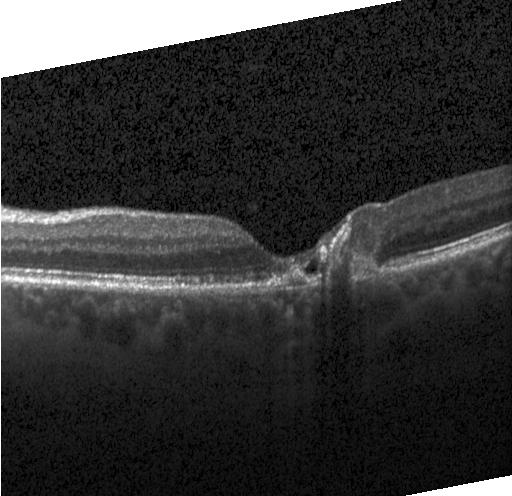

SD-OCT; instrument: Heidelberg Spectralis; horizontal scan through the fovea; OCT B-scan
Impression: a choroidal neovascular membrane.